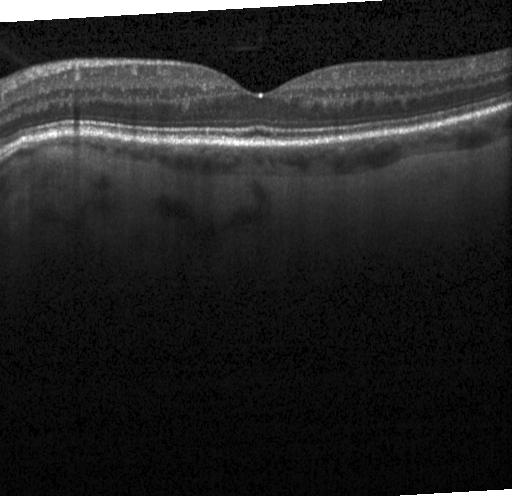
Impression: no choroidal neovascularization, no diabetic macular edema, and no drusen.